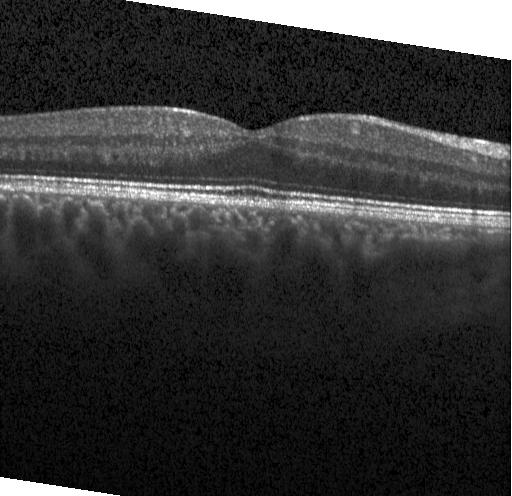 OCT line scan.
Assessment: neither CNV, DME, nor drusen.